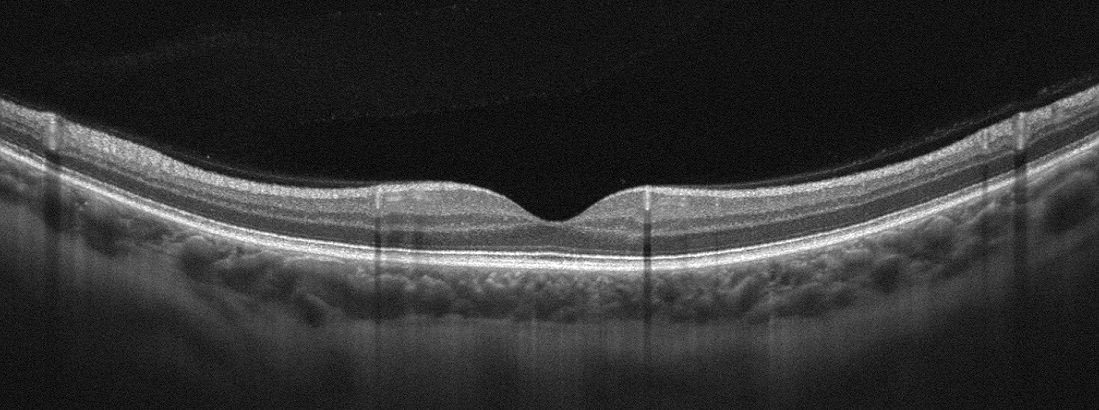 OCT line scan.
Diagnosis: no AMD, DME, ERM, RAO, RVO, or VID.